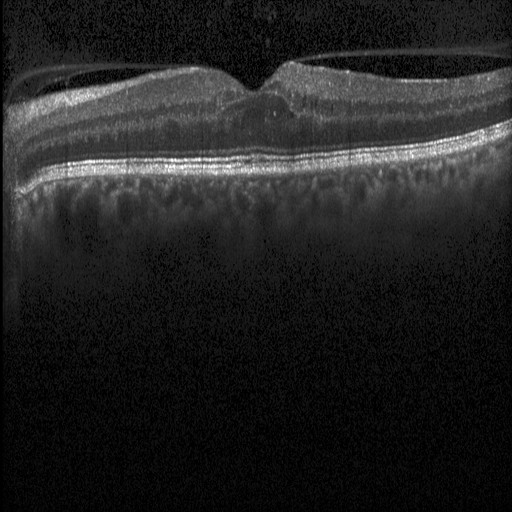

Spectral-domain optical coherence tomography; fovea-centered; Heidelberg Spectralis OCT system; OCT line scan
OCT finding: diabetic macular edema (DME).